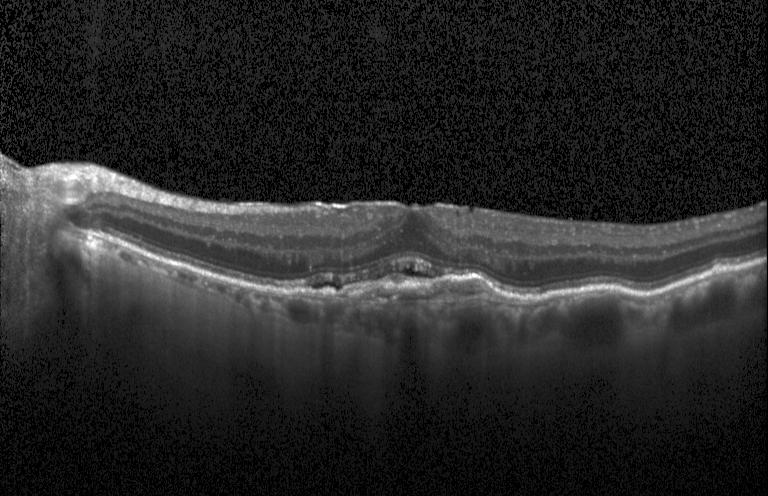
Heidelberg Spectralis OCT system, macular scan, retinal OCT cross-section, spectral-domain OCT
Macular OCT: CNV.